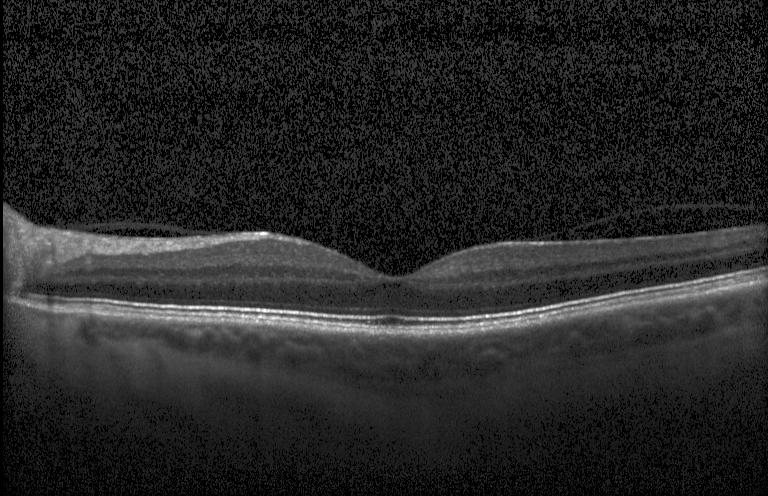
Optical coherence tomography scan, Heidelberg Spectralis — Macular OCT: no evidence of CNV, DME, or drusen.